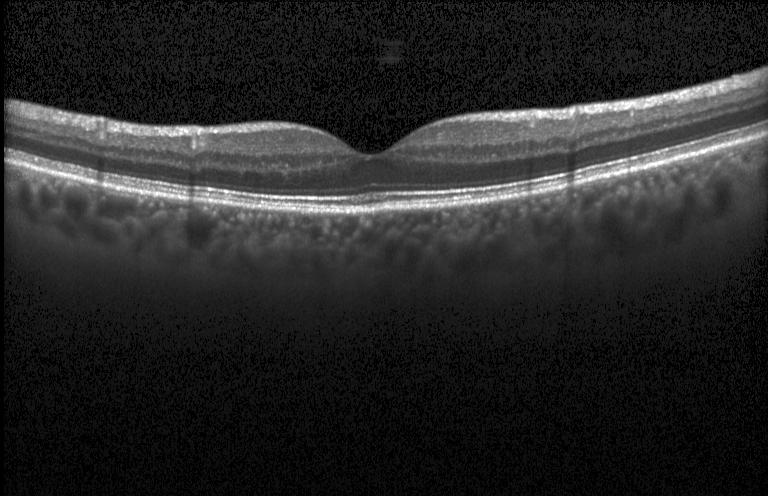
Retinal OCT B-scan. Horizontal scan through the fovea. SD-OCT. Heidelberg Spectralis OCT system.
Finding: neither CNV, DME, nor drusen.